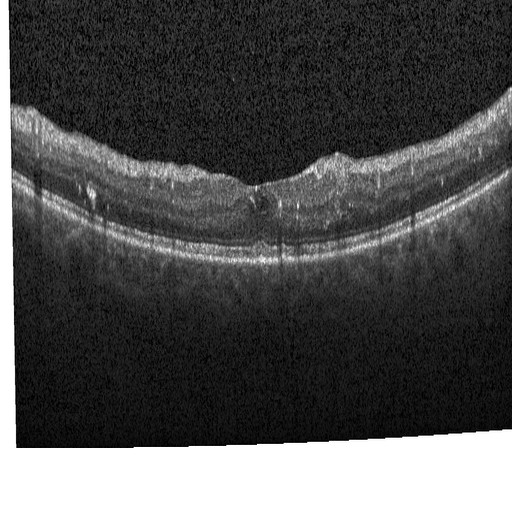 OCT B-scan showing diabetic macular edema (DME).